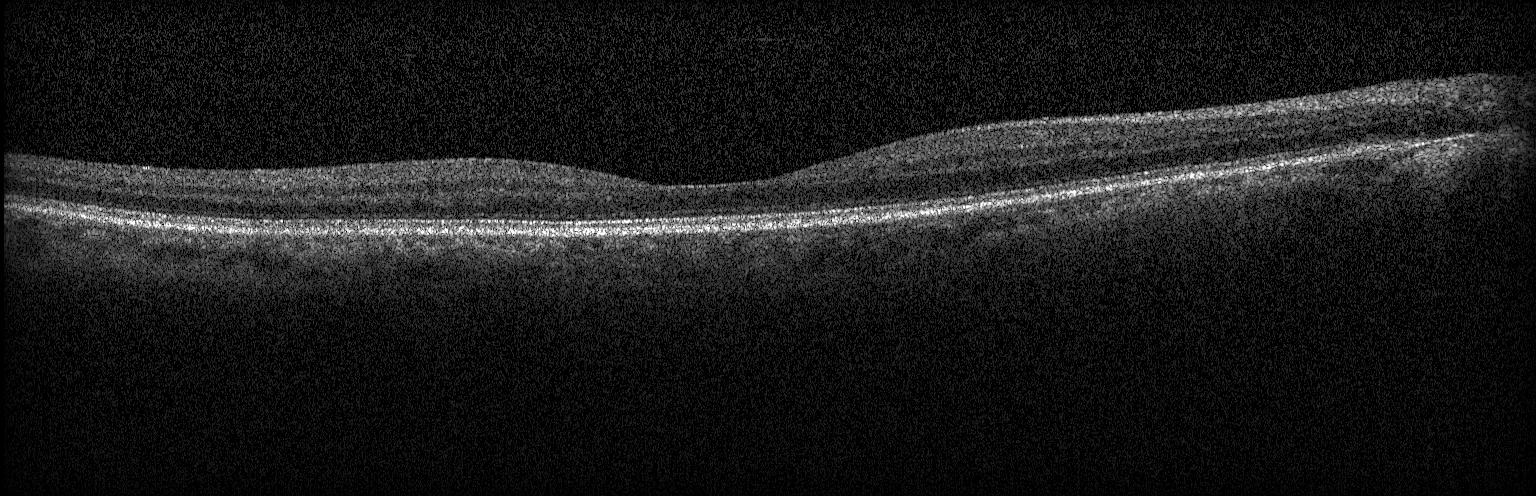

OCT line scan, acquired on a Heidelberg Spectralis, macular scan — Assessment: no CNV, DME, or drusen.